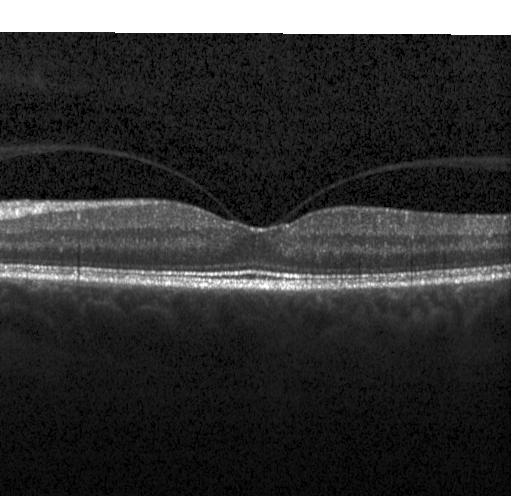

Heidelberg Spectralis · retinal OCT cross-section · centered on the fovea — Dx: neither choroidal neovascularization, diabetic macular edema, nor drusen.